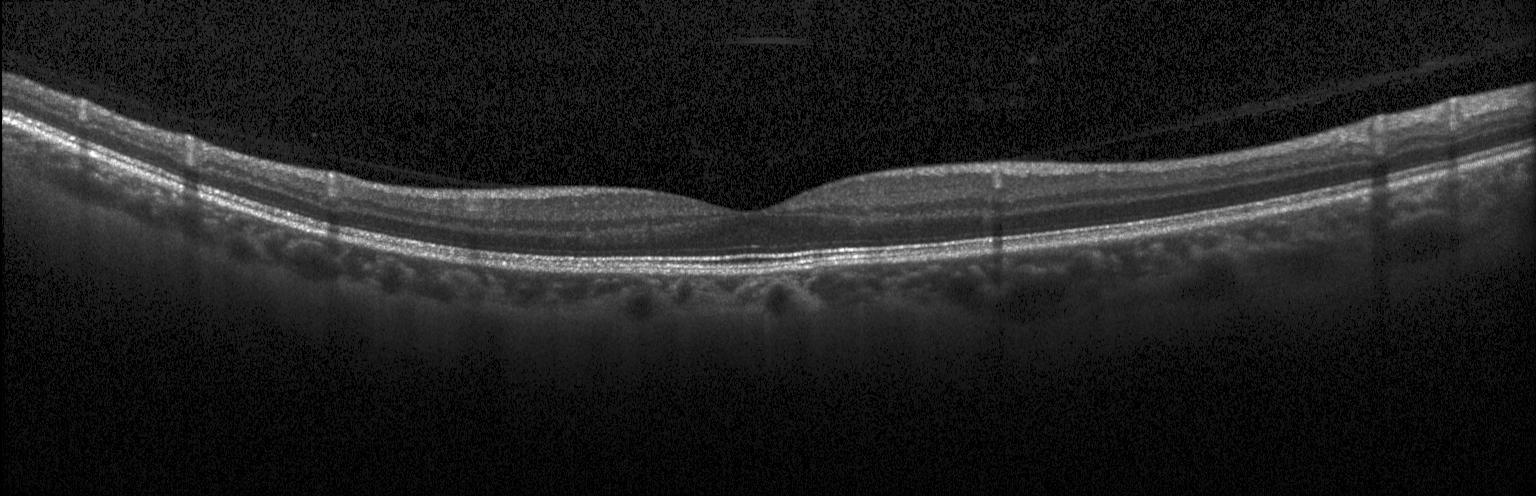

Retinal OCT B-scan. OCT finding: no choroidal neovascularization, diabetic macular edema, or drusen.